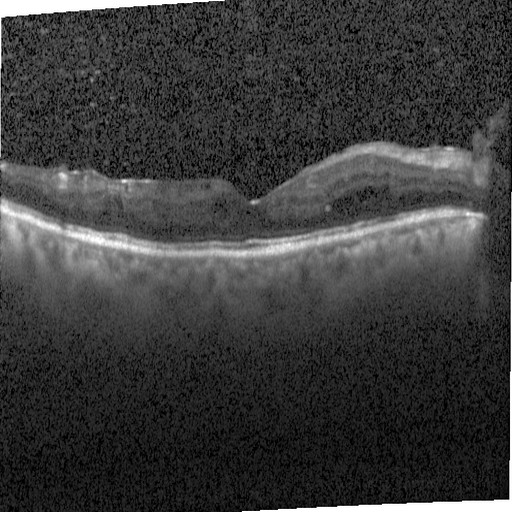
Centered on the fovea; spectral-domain optical coherence tomography; instrument: Heidelberg Spectralis; retinal OCT cross-section.
Impression: DME.